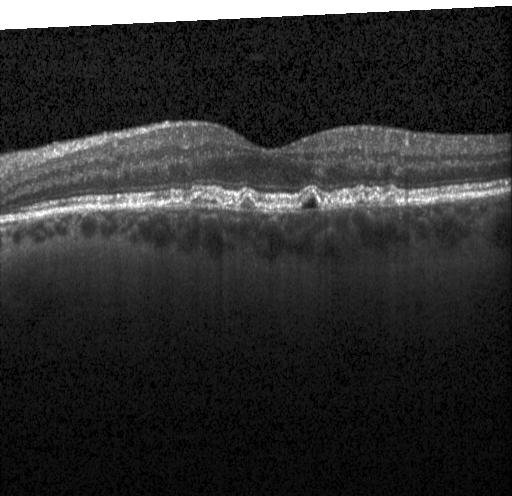
Macular OCT: sub-RPE drusenoid deposits.